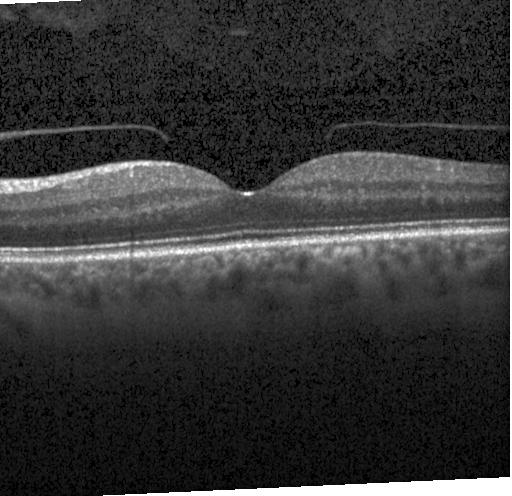

SD-OCT. Acquired on a Heidelberg Spectralis. Through the macula. Retinal OCT cross-section.
Impression: neither choroidal neovascularization, diabetic macular edema, nor drusen.